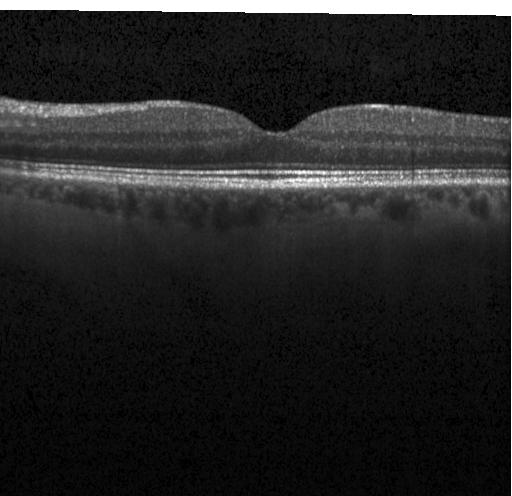 OCT line scan. Spectral-domain optical coherence tomography. Fovea-centered. Heidelberg Spectralis OCT system.
Diagnosis: no CNV, DME, or drusen.